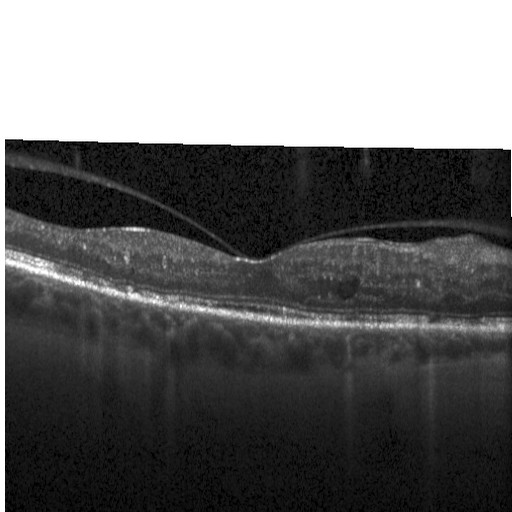

Optical coherence tomography B-scan; acquired on a Heidelberg Spectralis; spectral-domain OCT; centered on the fovea.
Diabetic macular edema.